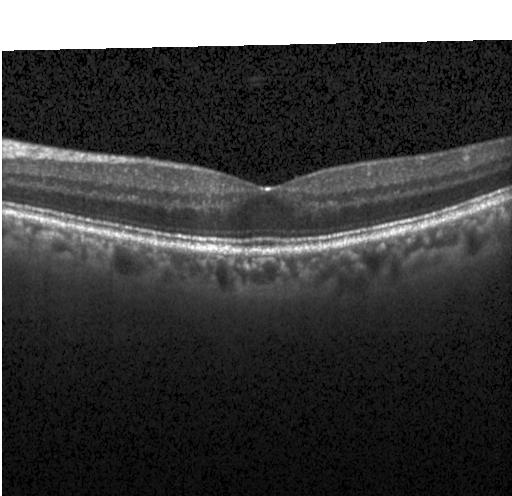 Through the macula · SD-OCT · optical coherence tomography scan · Heidelberg Spectralis OCT system — Finding: neither choroidal neovascularization, diabetic macular edema, nor drusen.